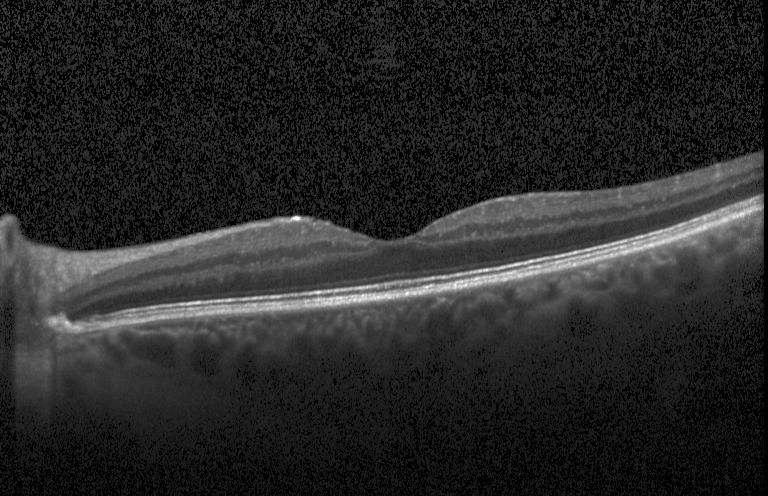
Finding: no choroidal neovascularization, no diabetic macular edema, and no drusen.